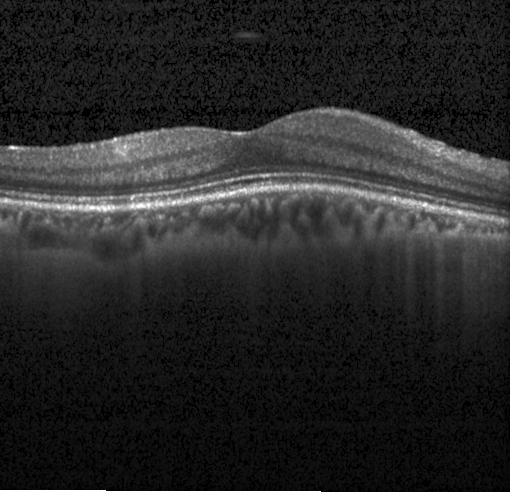
Macular OCT demonstrating no choroidal neovascularization, no diabetic macular edema, and no drusen.